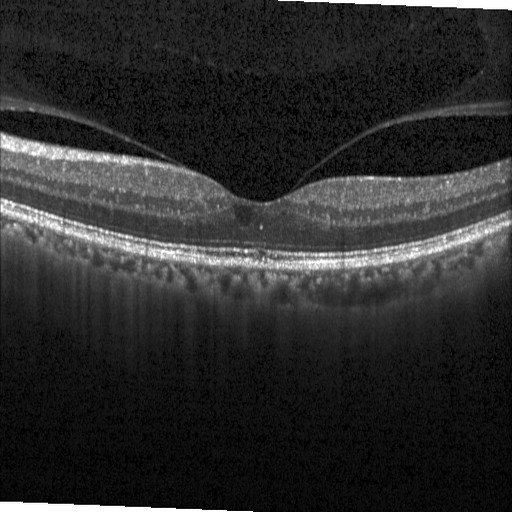

Finding: diabetic macular edema (DME).